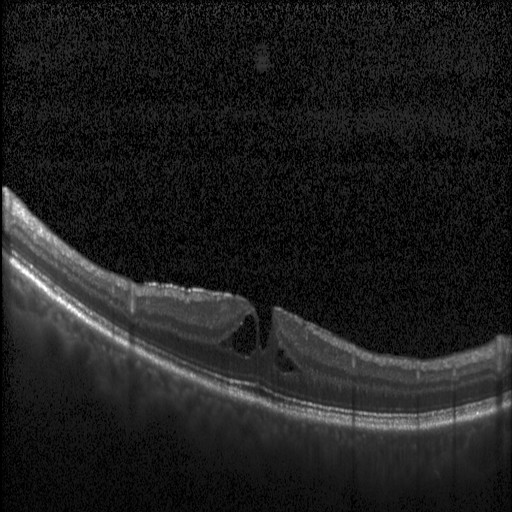 Retinal OCT cross-section, fovea-centered
Impression: DME.